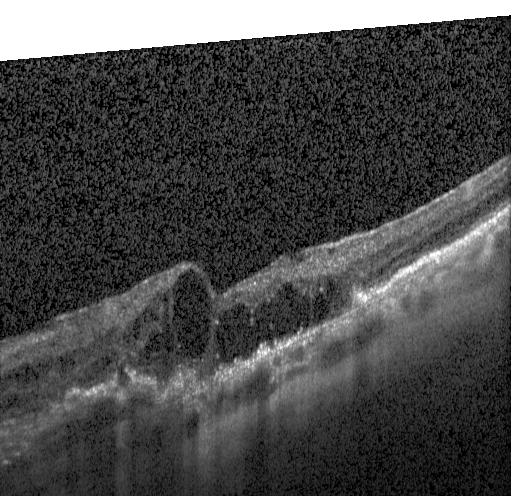 Retinal OCT B-scan; spectral-domain optical coherence tomography. A choroidal neovascular membrane.